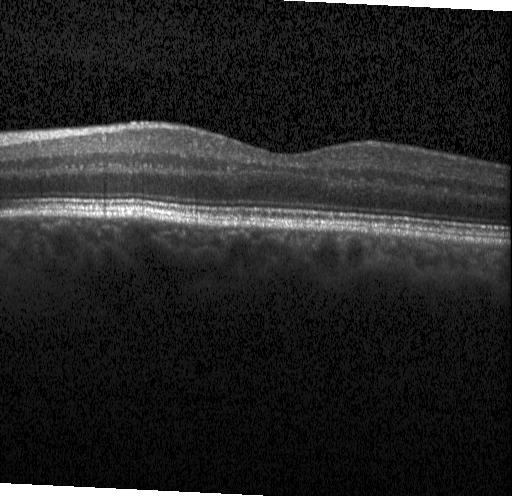
Spectral-domain OCT, instrument: Heidelberg Spectralis, through the macula, retinal OCT cross-section
Diagnosis: no evidence of choroidal neovascularization, diabetic macular edema, or drusen.